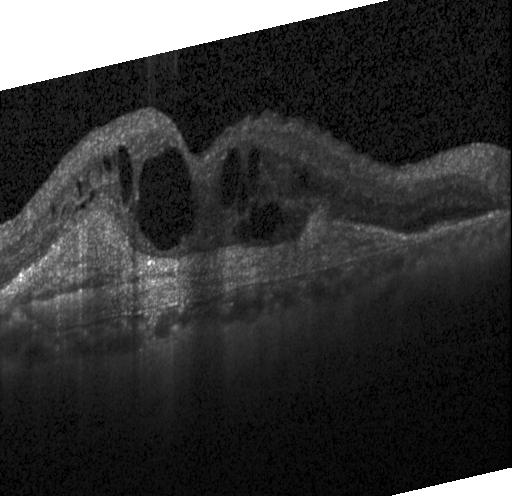

OCT line scan
This B-scan demonstrates CNV.